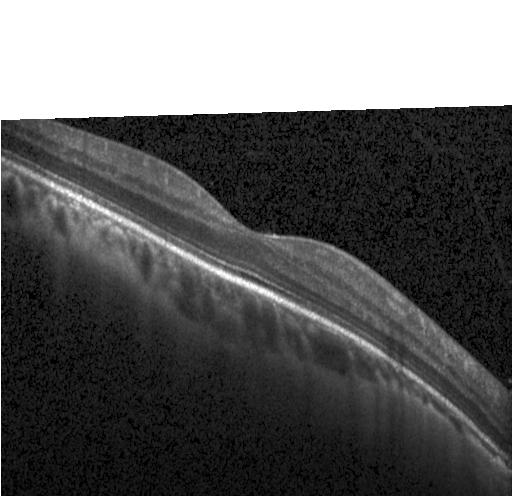

Retinal OCT cross-section showing no choroidal neovascularization, no diabetic macular edema, and no drusen.